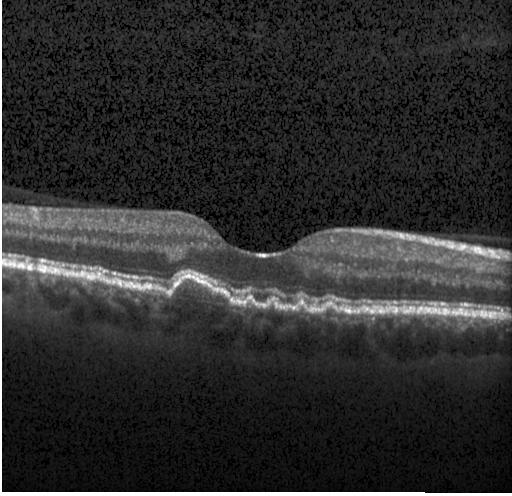 This B-scan demonstrates sub-RPE drusenoid deposits.